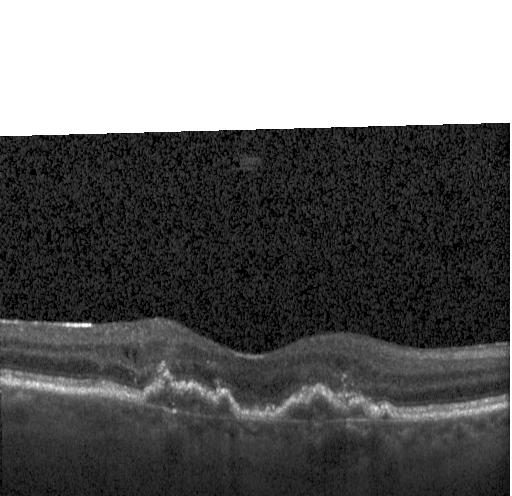
OCT B-scan. Dx: CNV.